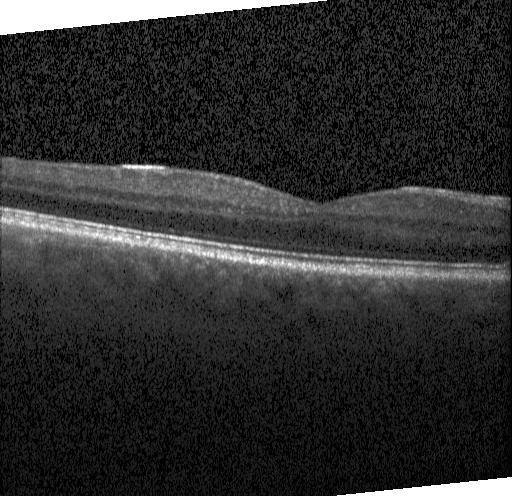

OCT finding: no CNV, no DME, and no drusen.